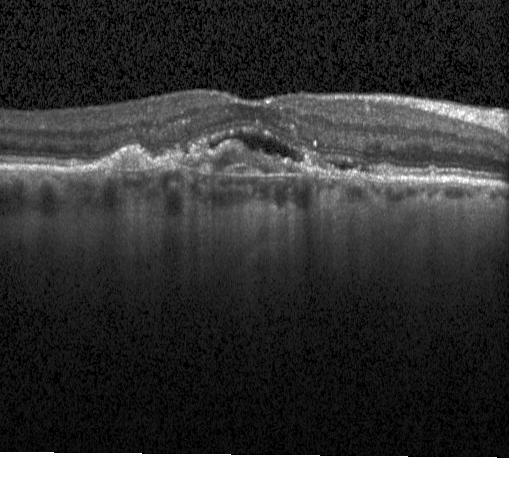

Horizontal scan through the fovea, spectral-domain optical coherence tomography, OCT B-scan, Heidelberg Spectralis
Impression: a choroidal neovascular membrane.